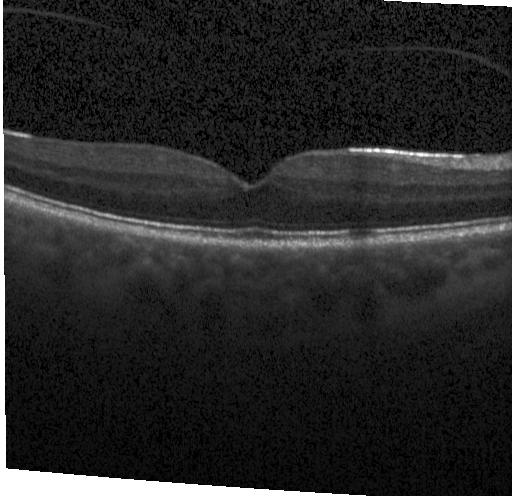
Retinal OCT cross-section.
No choroidal neovascularization, diabetic macular edema, or drusen.